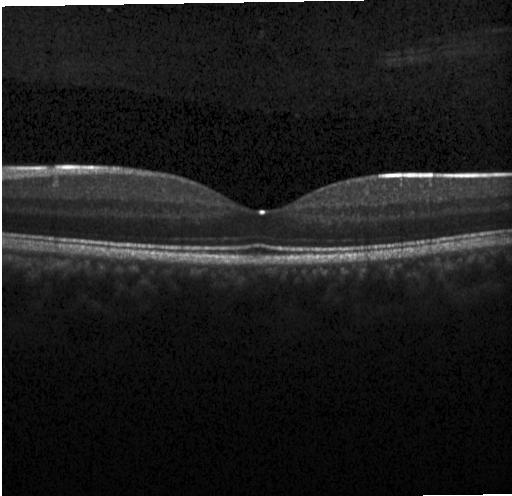 No evidence of choroidal neovascularization, diabetic macular edema, or drusen.